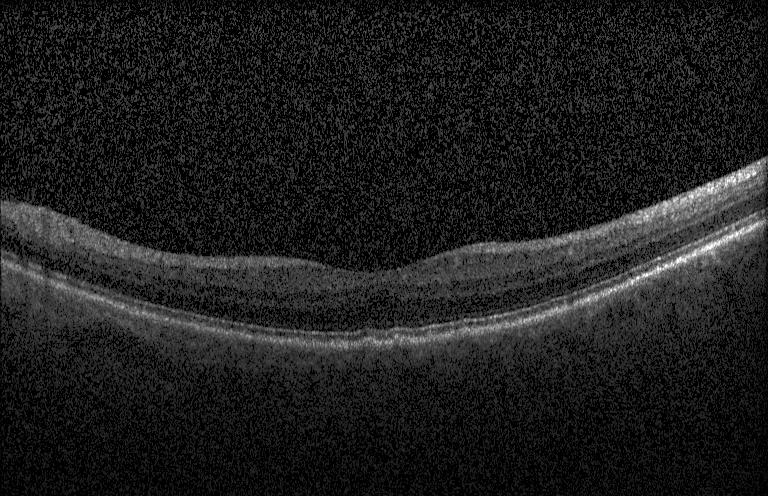 Retinal OCT cross-section. Finding: sub-RPE drusenoid deposits.